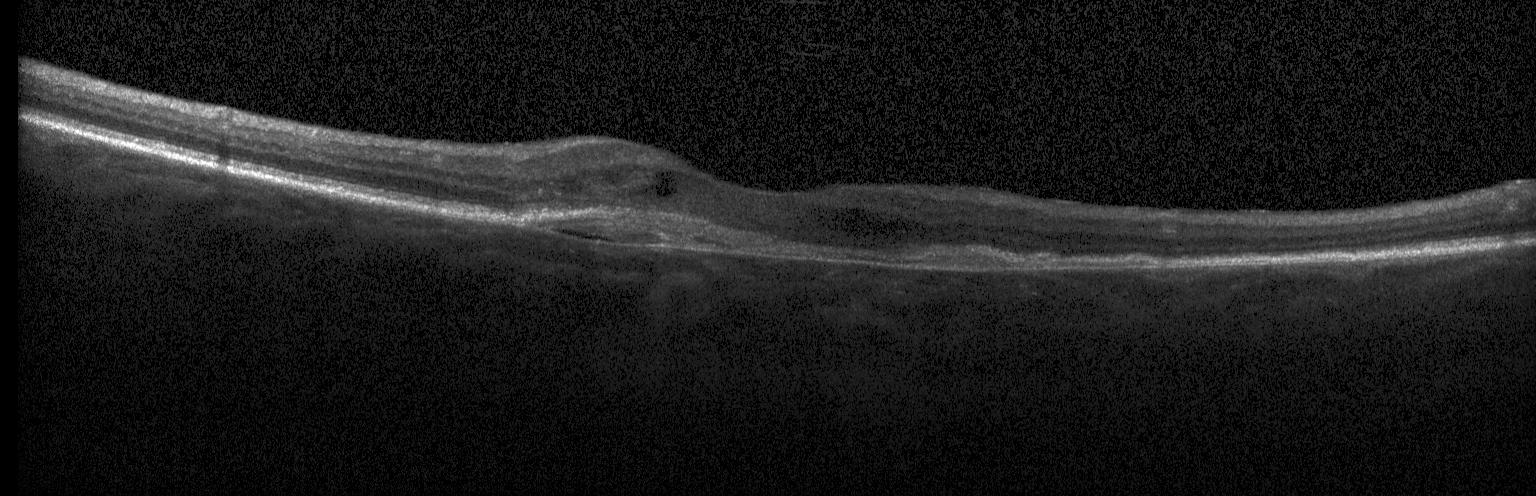 Optical coherence tomography scan, spectral-domain optical coherence tomography, horizontal scan through the fovea, Heidelberg Spectralis. Dx: a choroidal neovascular membrane.